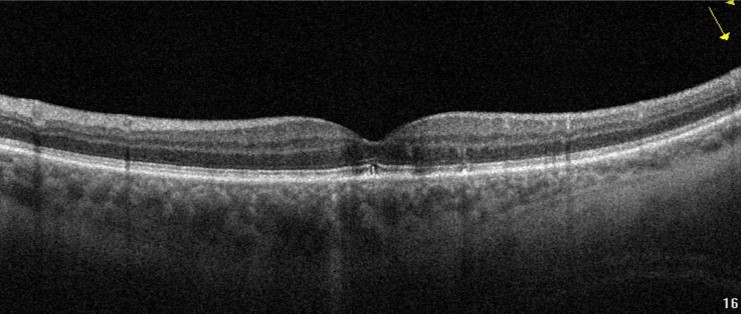

Optical coherence tomography scan. Instrument: Optovue Avanti RTVue XR. Macular scan — Diagnosis: AMD.